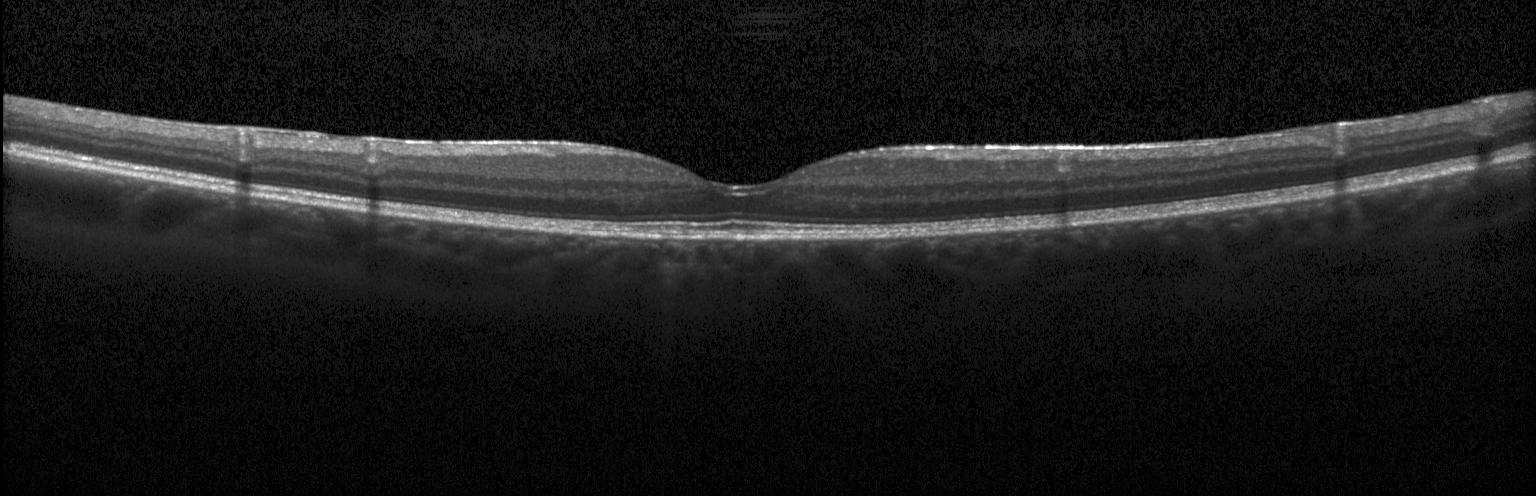 Horizontal scan through the fovea, Heidelberg Spectralis, retinal OCT cross-section, SD-OCT.
No choroidal neovascularization, no diabetic macular edema, and no drusen.